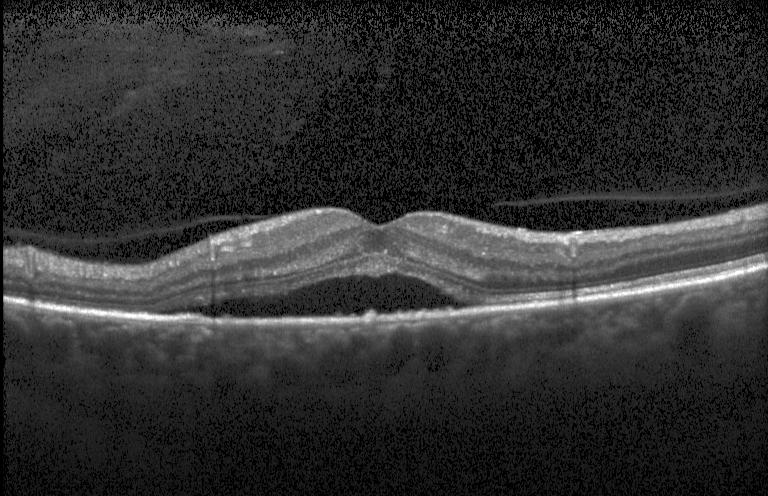
Fovea-centered · optical coherence tomography scan
Impression: a choroidal neovascular membrane.